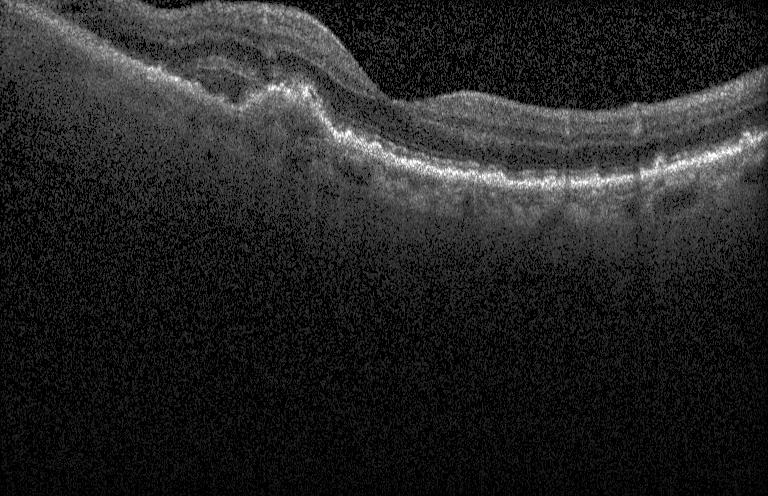
Fovea-centered, spectral-domain OCT, retinal OCT cross-section, Heidelberg Spectralis.
Assessment: a choroidal neovascular membrane.